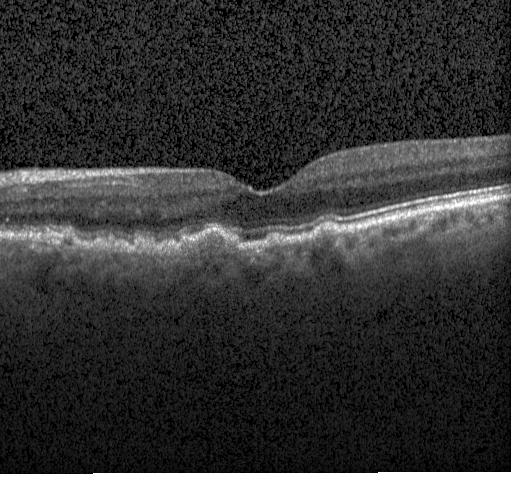 Optical coherence tomography B-scan; centered on the fovea — Finding: multiple drusen.